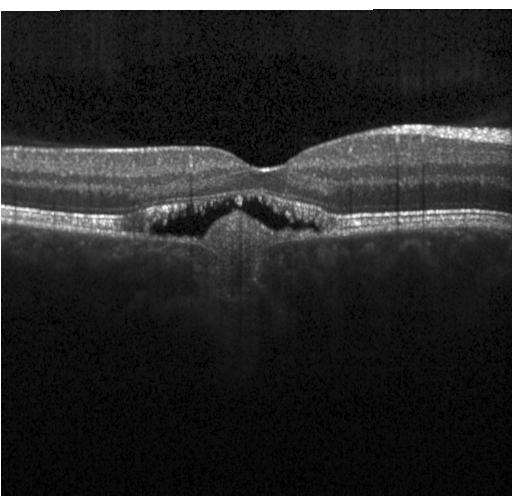 Finding: a choroidal neovascular membrane.